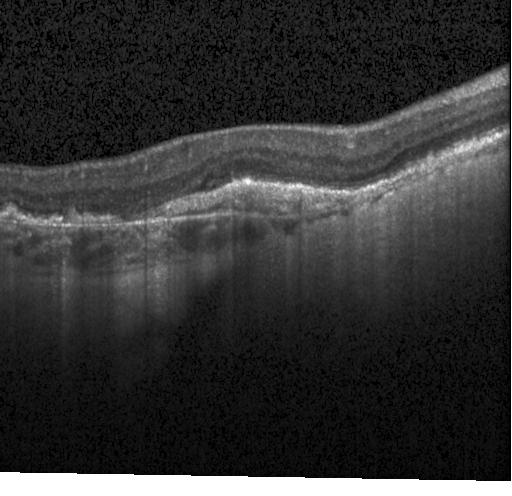 Retinal OCT cross-section — Diagnosis: a choroidal neovascular membrane.